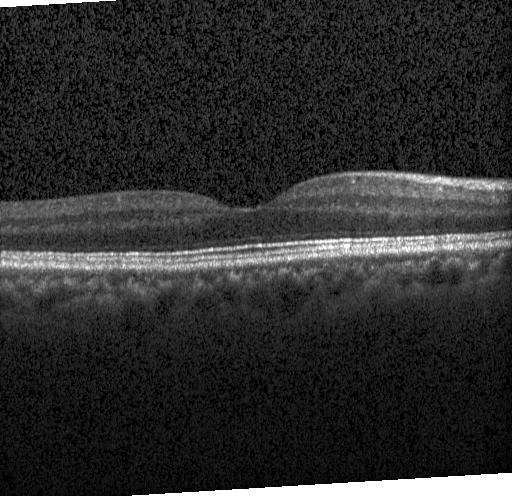 Macular scan. SD-OCT. Optical coherence tomography scan.
Diagnosis: no evidence of choroidal neovascularization, diabetic macular edema, or drusen.